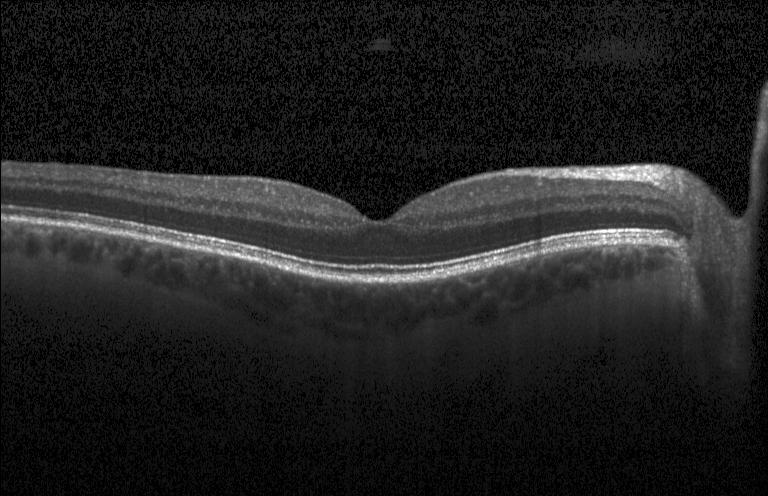
Spectral-domain OCT B-scan: no choroidal neovascularization, diabetic macular edema, or drusen.